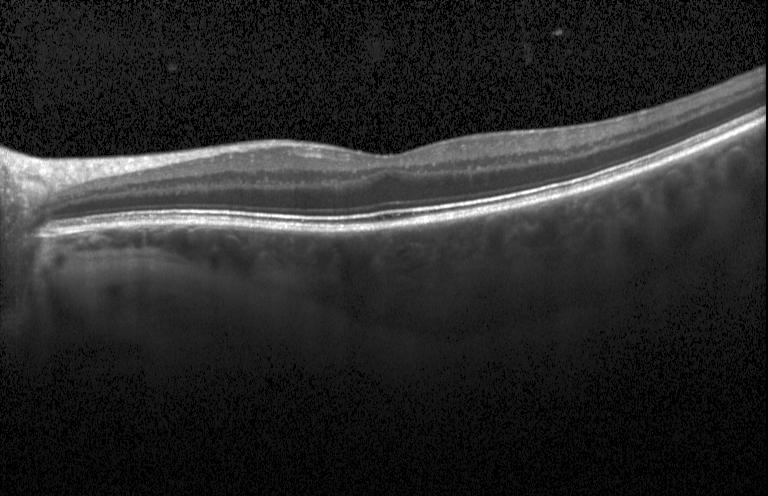
Acquired on a Heidelberg Spectralis. Retinal OCT cross-section. Fovea-centered. Spectral-domain OCT — Finding: no evidence of CNV, DME, or drusen.